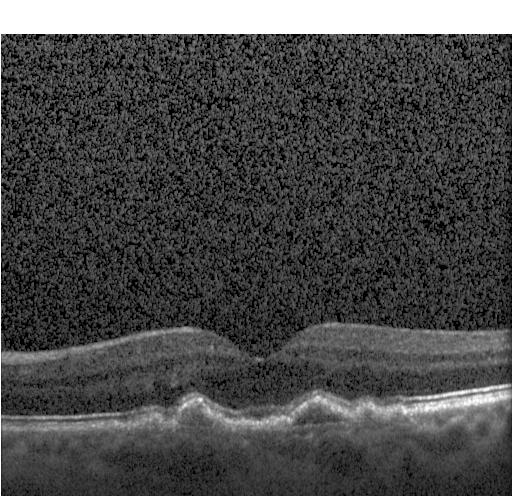
Sub-RPE drusenoid deposits.